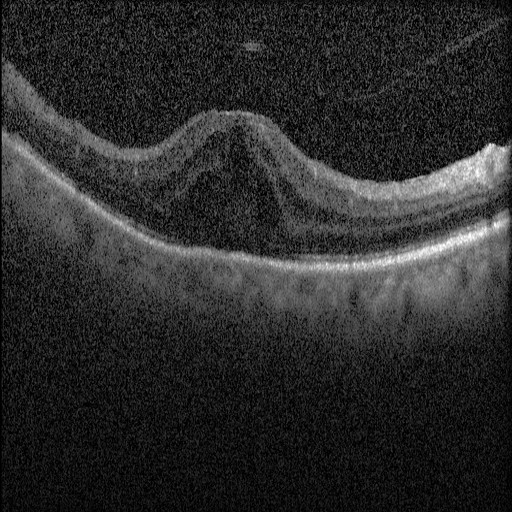 Impression: diabetic macular edema.